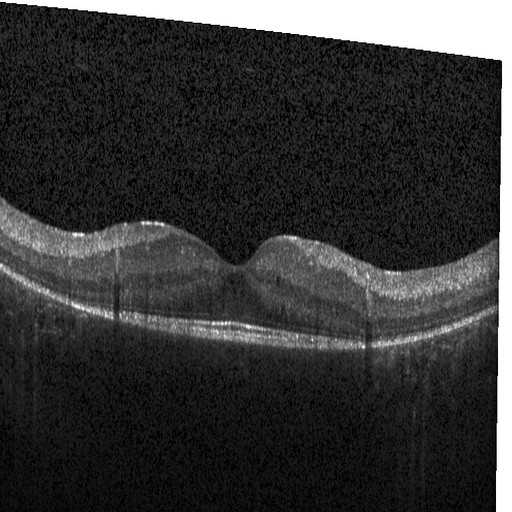
Optical coherence tomography B-scan — Assessment: DME.